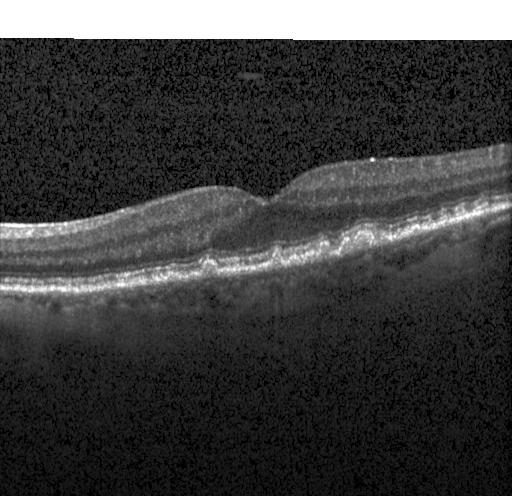

Assessment: sub-RPE drusenoid deposits.